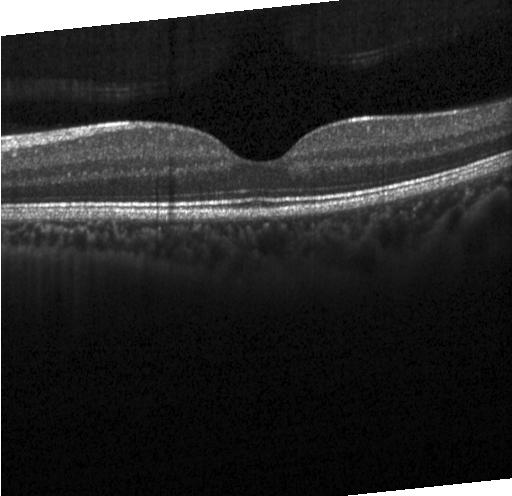

SD-OCT · retinal OCT B-scan. Dx: no evidence of choroidal neovascularization, diabetic macular edema, or drusen.